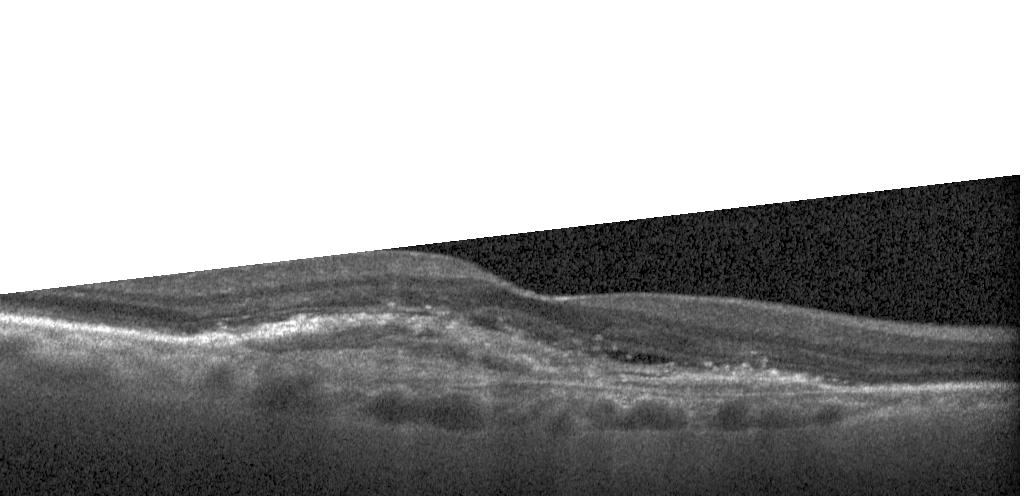 OCT scan showing a choroidal neovascular membrane.